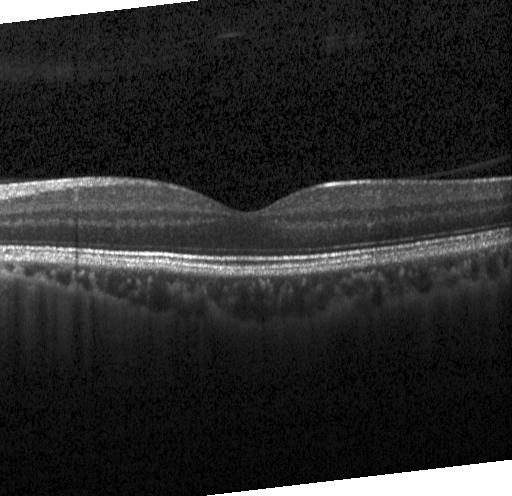 Through the macula; instrument: Heidelberg Spectralis; retinal OCT cross-section
No choroidal neovascularization, diabetic macular edema, or drusen.